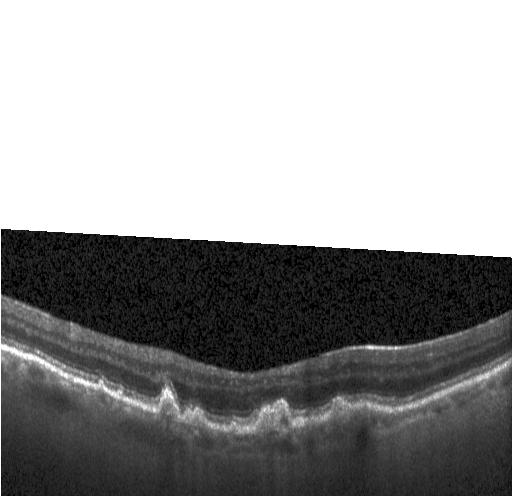 Dx: multiple drusen.